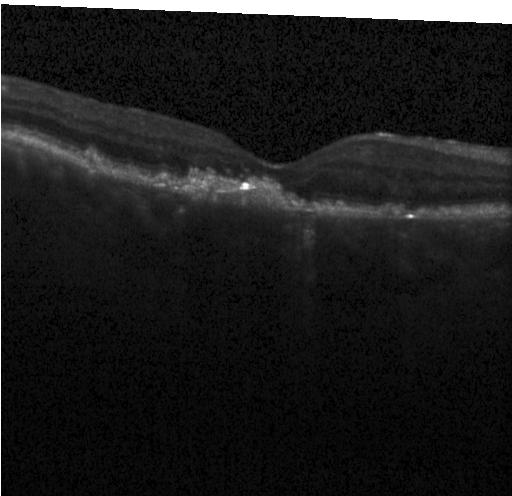
Retinal OCT cross-section showing a choroidal neovascular membrane.